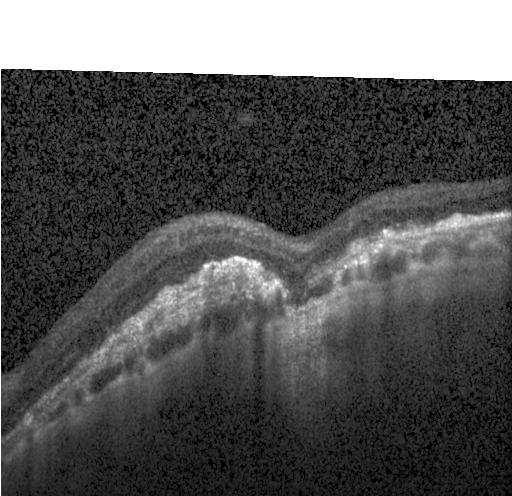 OCT finding: a choroidal neovascular membrane.